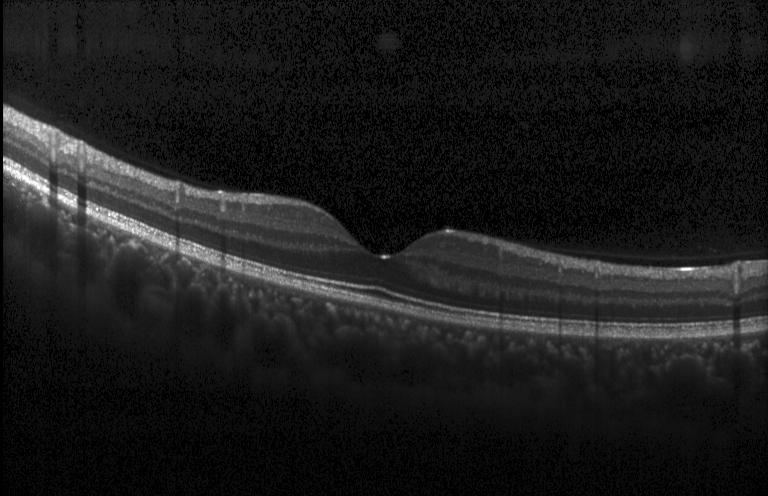 Fovea-centered · OCT line scan · Heidelberg Spectralis · spectral-domain optical coherence tomography. The scan shows no choroidal neovascularization, no diabetic macular edema, and no drusen.